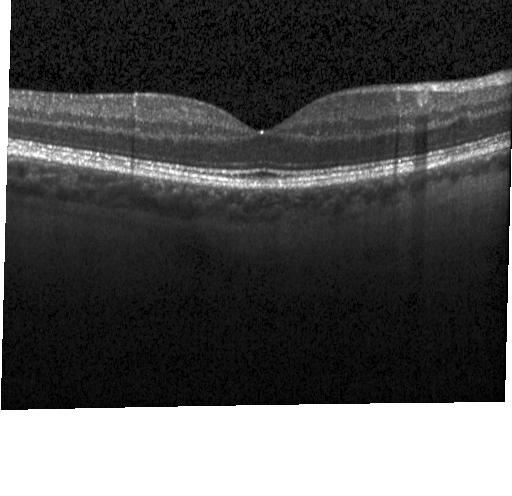 The scan shows no choroidal neovascularization, diabetic macular edema, or drusen.